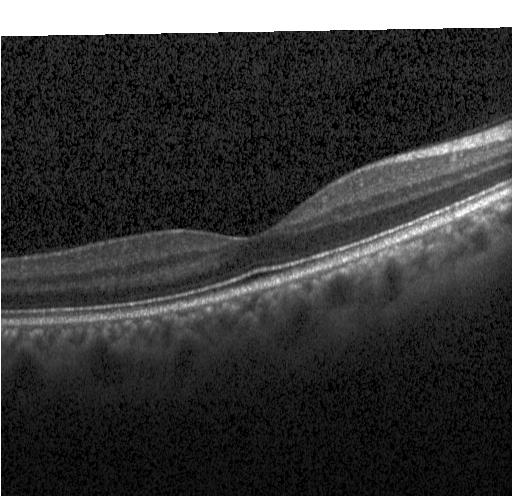
Horizontal scan through the fovea, OCT line scan, Heidelberg Spectralis OCT system — This B-scan demonstrates no choroidal neovascularization, no diabetic macular edema, and no drusen.